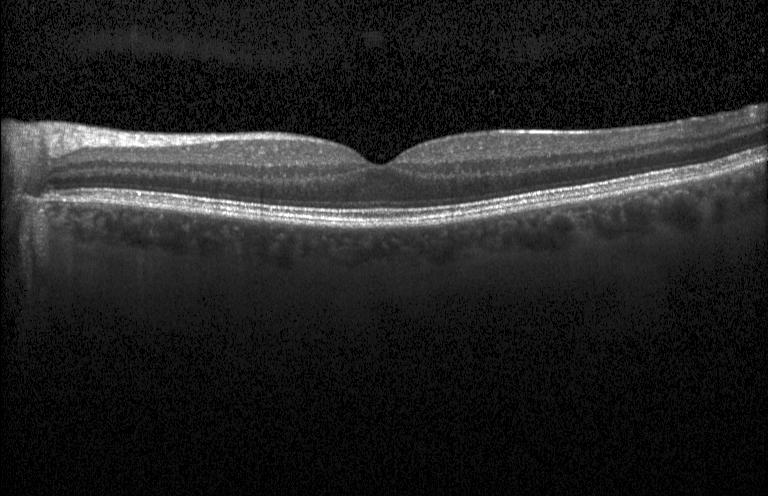
Acquired on a Heidelberg Spectralis · OCT line scan. Impression: no choroidal neovascularization, no diabetic macular edema, and no drusen.